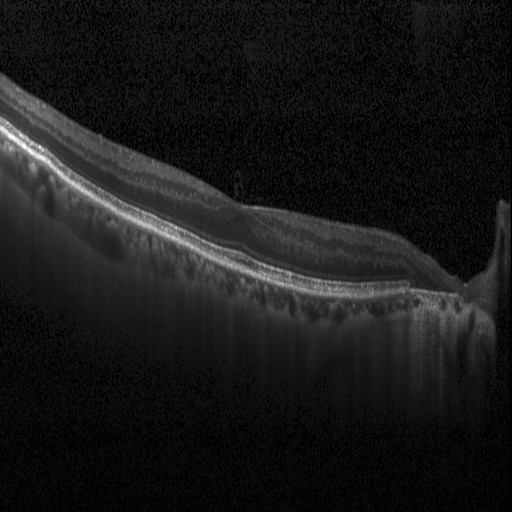 OCT scan showing diabetic macular edema (DME).